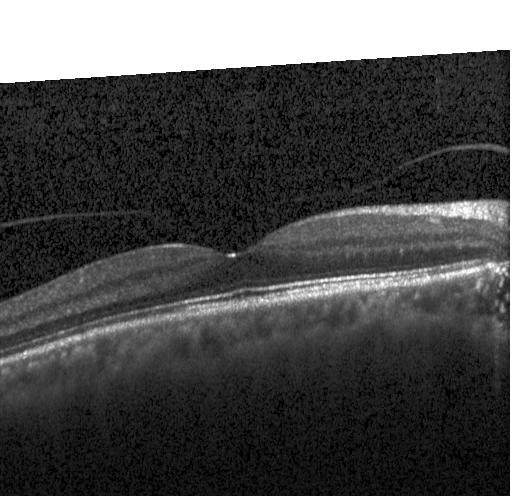

Diagnosis: no choroidal neovascularization, diabetic macular edema, or drusen.